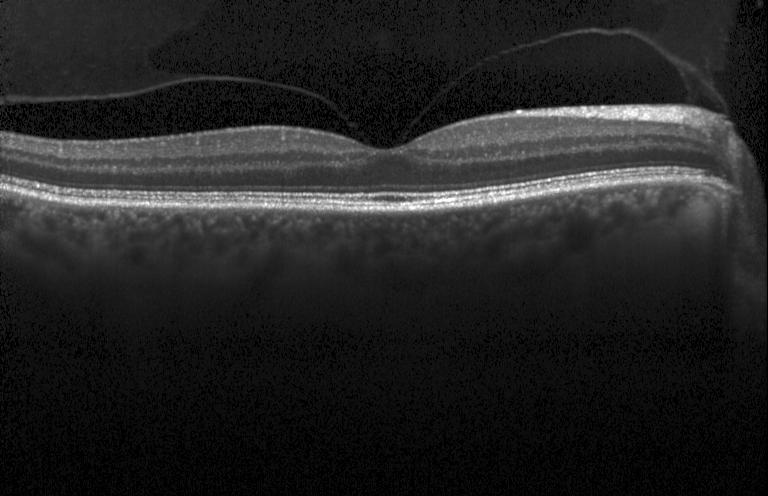 OCT B-scan. OCT finding: no CNV, no DME, and no drusen.